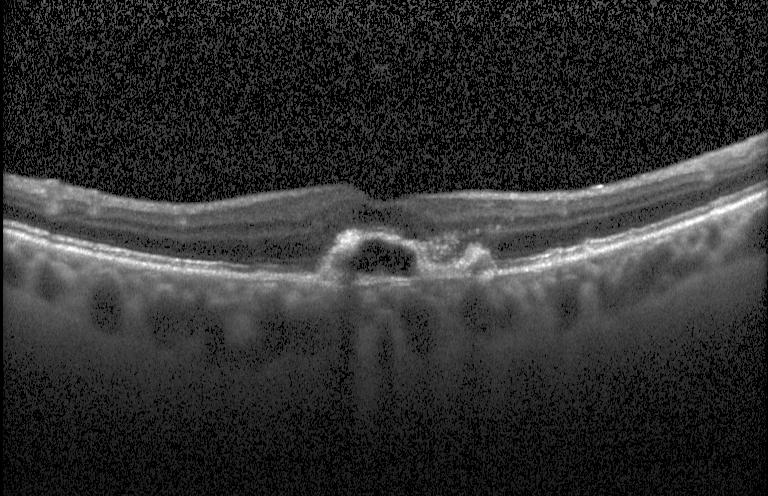 Through the macula · instrument: Heidelberg Spectralis · SD-OCT · optical coherence tomography B-scan
Diagnosis: a choroidal neovascular membrane.